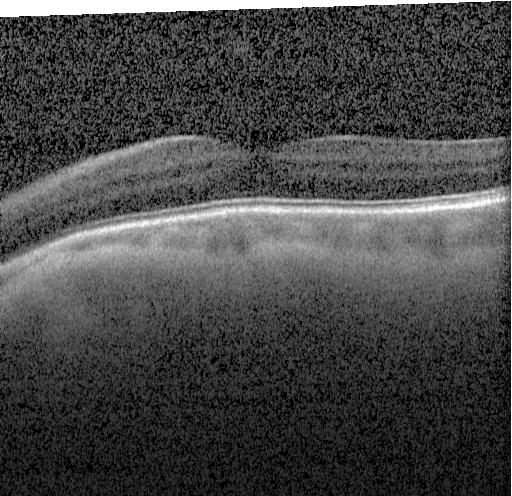

OCT B-scan showing neither choroidal neovascularization, diabetic macular edema, nor drusen.